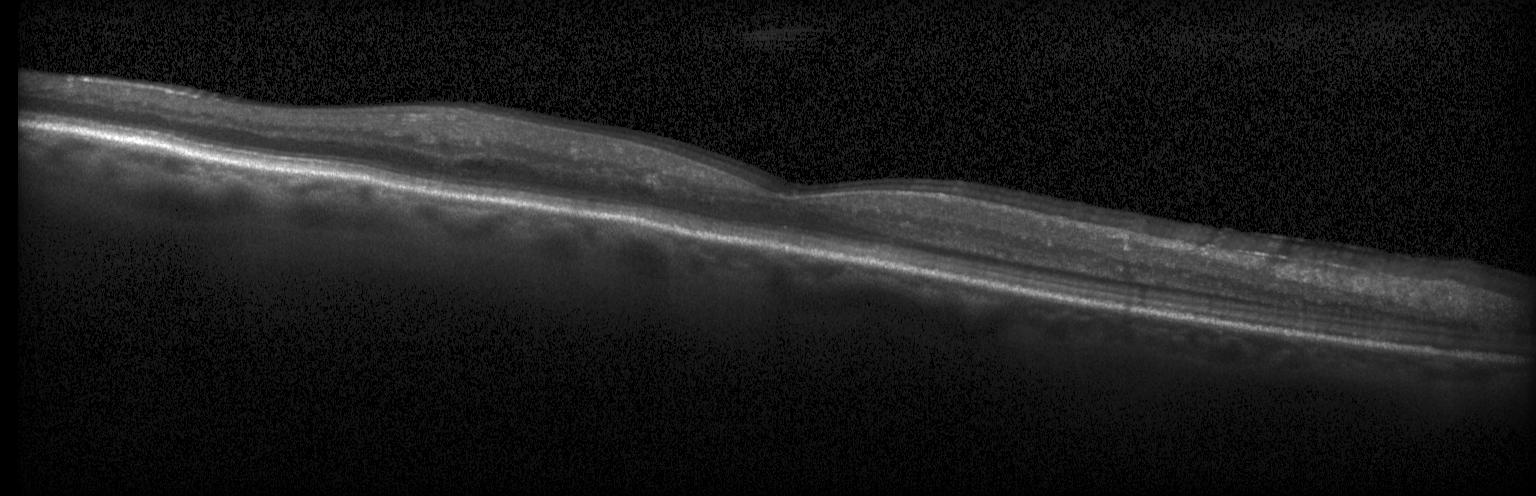
Macular OCT: no evidence of CNV, DME, or drusen.